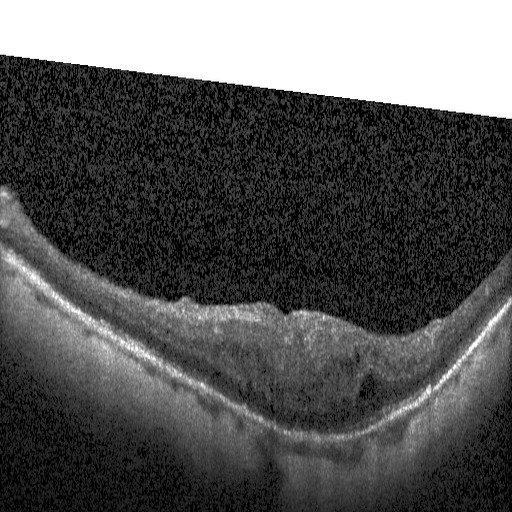

Spectral-domain OCT · instrument: Heidelberg Spectralis · through the macula · OCT line scan.
Diagnosis: diabetic macular edema.